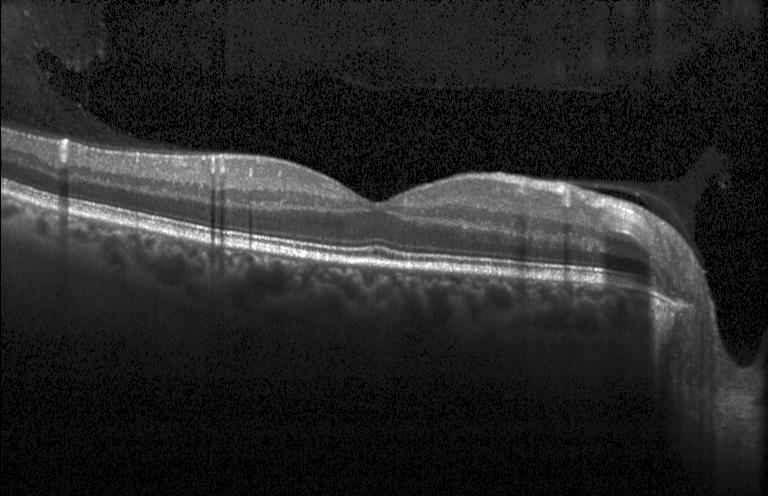 Retinal OCT cross-section
This B-scan demonstrates neither CNV, DME, nor drusen.